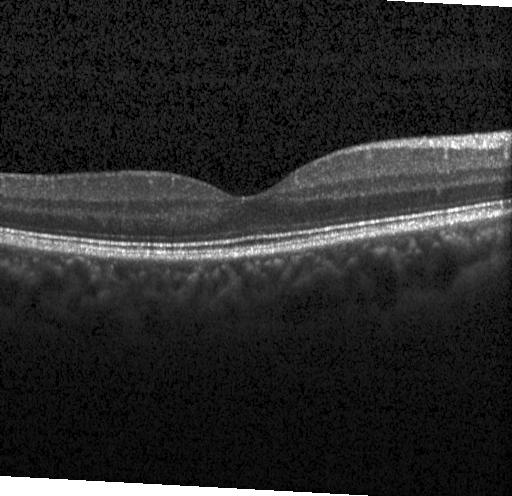

Heidelberg Spectralis OCT system, through the macula, OCT B-scan.
This B-scan demonstrates no evidence of CNV, DME, or drusen.